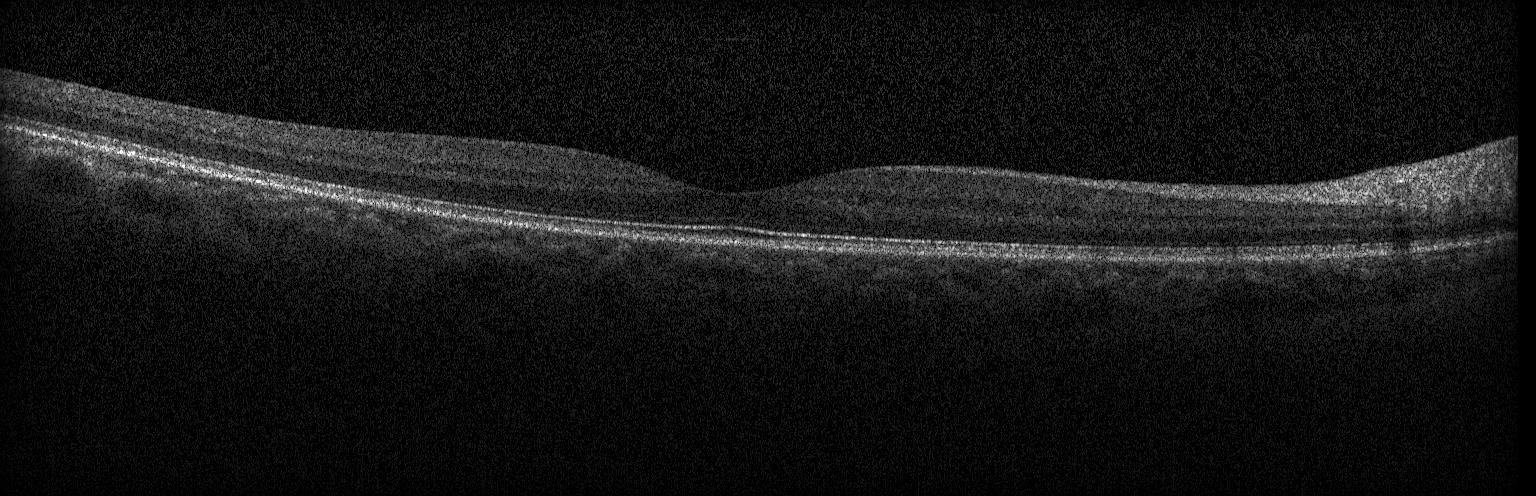

OCT B-scan.
Finding: no evidence of choroidal neovascularization, diabetic macular edema, or drusen.